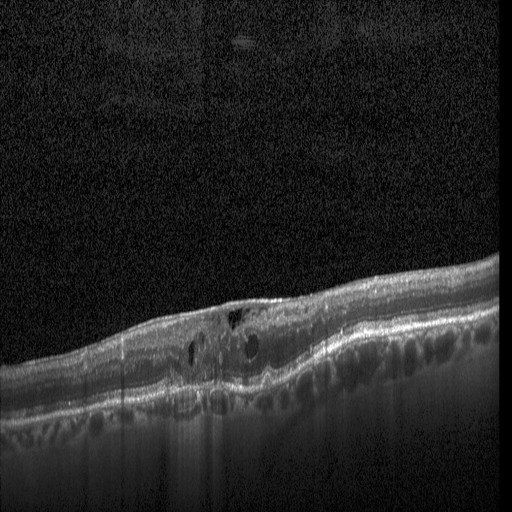

Diagnosis: diabetic macular edema.